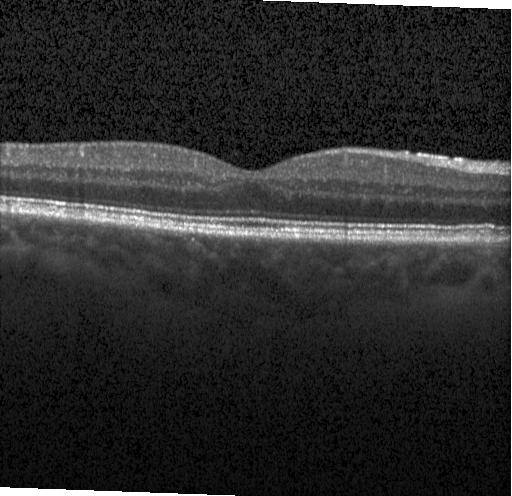
Retinal OCT cross-section. OCT finding: no choroidal neovascularization, diabetic macular edema, or drusen.